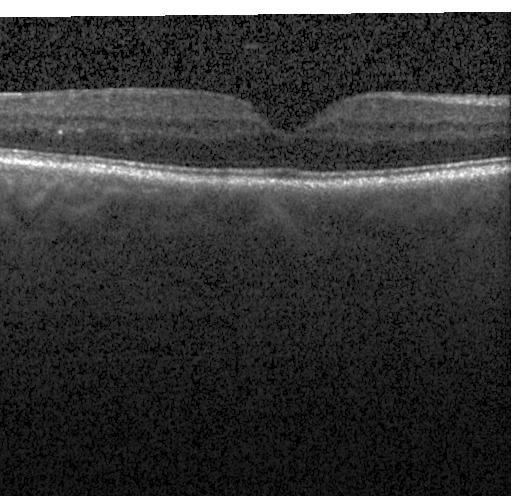 Optical coherence tomography scan.
OCT finding: no evidence of choroidal neovascularization, diabetic macular edema, or drusen.